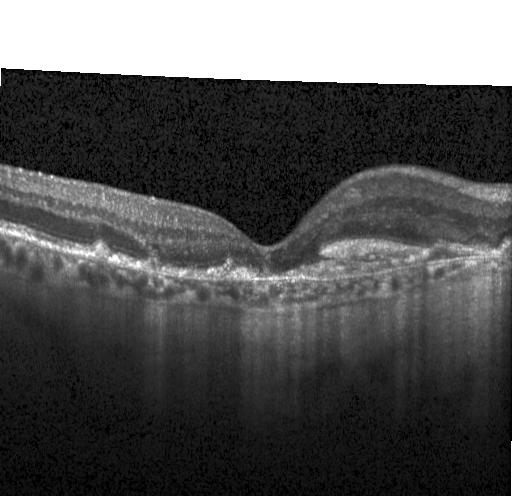
Macular OCT demonstrating choroidal neovascularization (CNV).